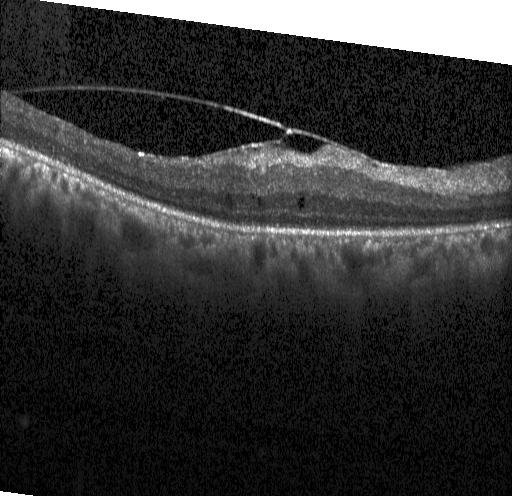 Optical coherence tomography scan · spectral-domain optical coherence tomography · Heidelberg Spectralis.
Assessment: diabetic macular edema (DME).